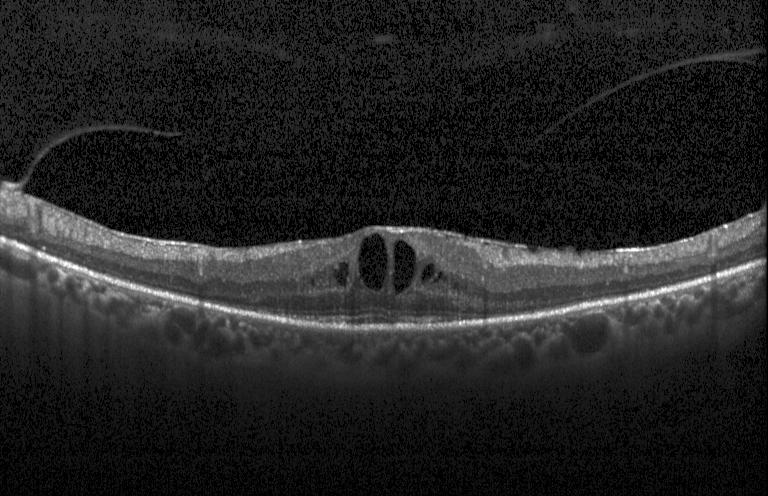

OCT line scan. Horizontal scan through the fovea. OCT finding: diabetic macular edema (DME).